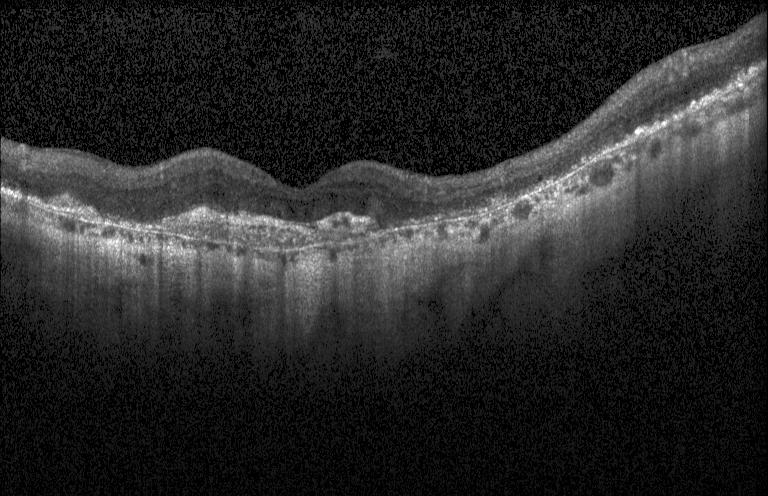 OCT B-scan. SD-OCT — OCT finding: a choroidal neovascular membrane.